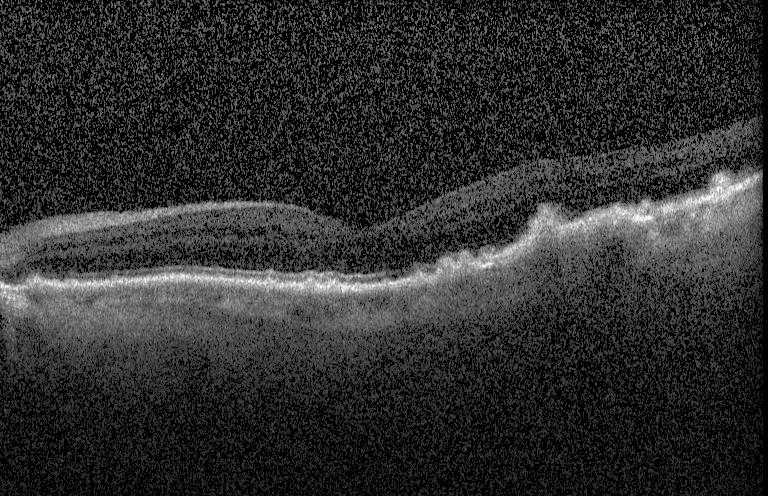 Macular scan · spectral-domain optical coherence tomography · retinal OCT cross-section. Dx: a choroidal neovascular membrane.